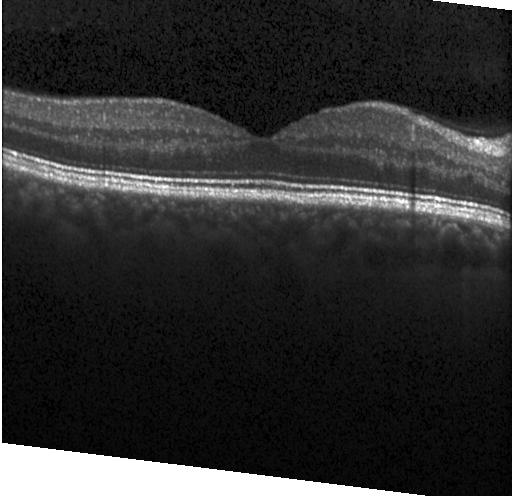

Macular OCT demonstrating no evidence of CNV, DME, or drusen.